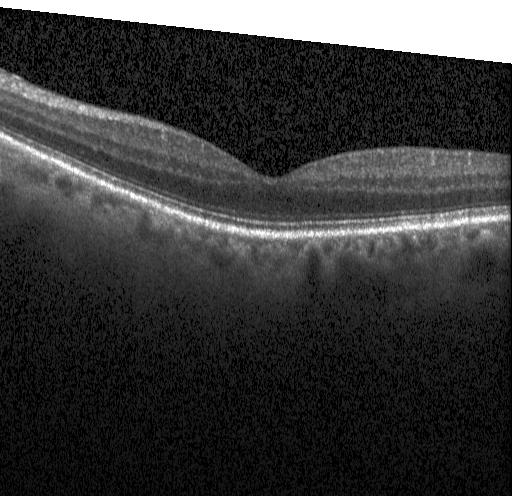
Finding: neither CNV, DME, nor drusen.